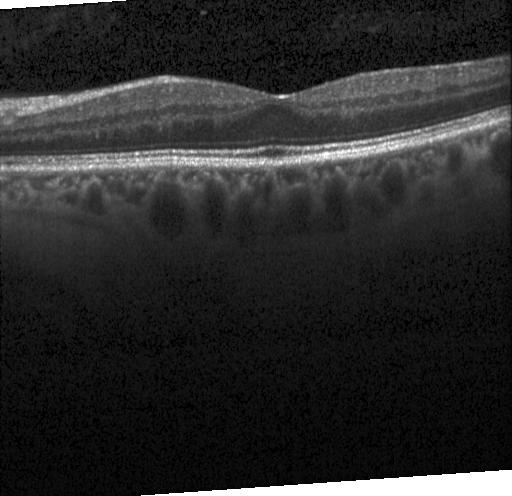 Retinal OCT cross-section · spectral-domain OCT · Heidelberg Spectralis OCT system. Impression: no CNV, DME, or drusen.